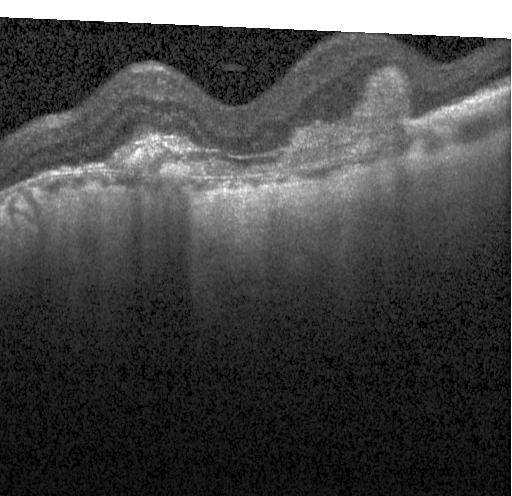
The scan shows a choroidal neovascular membrane.